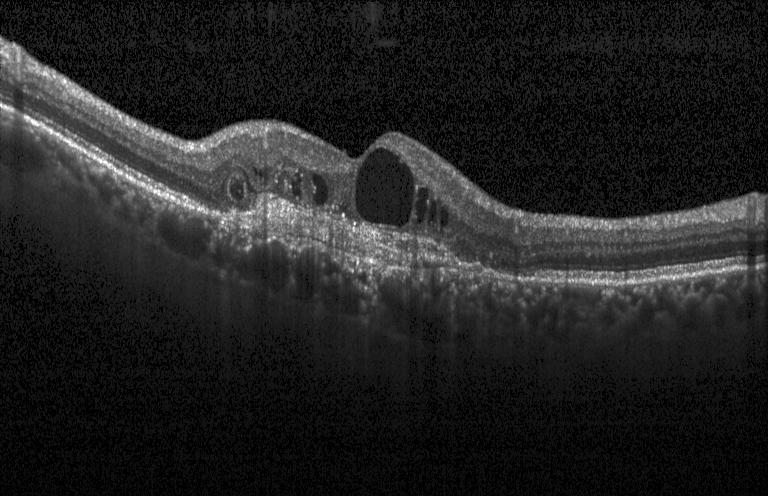

This B-scan demonstrates choroidal neovascularization.